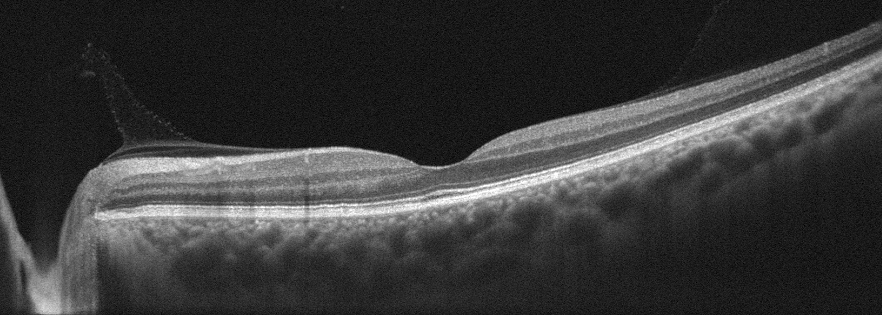 Retinal OCT cross-section · macular scan · left eye · instrument: Optovue Avanti RTVue XR.
No AMD, DME, ERM, RAO, RVO, or VID.